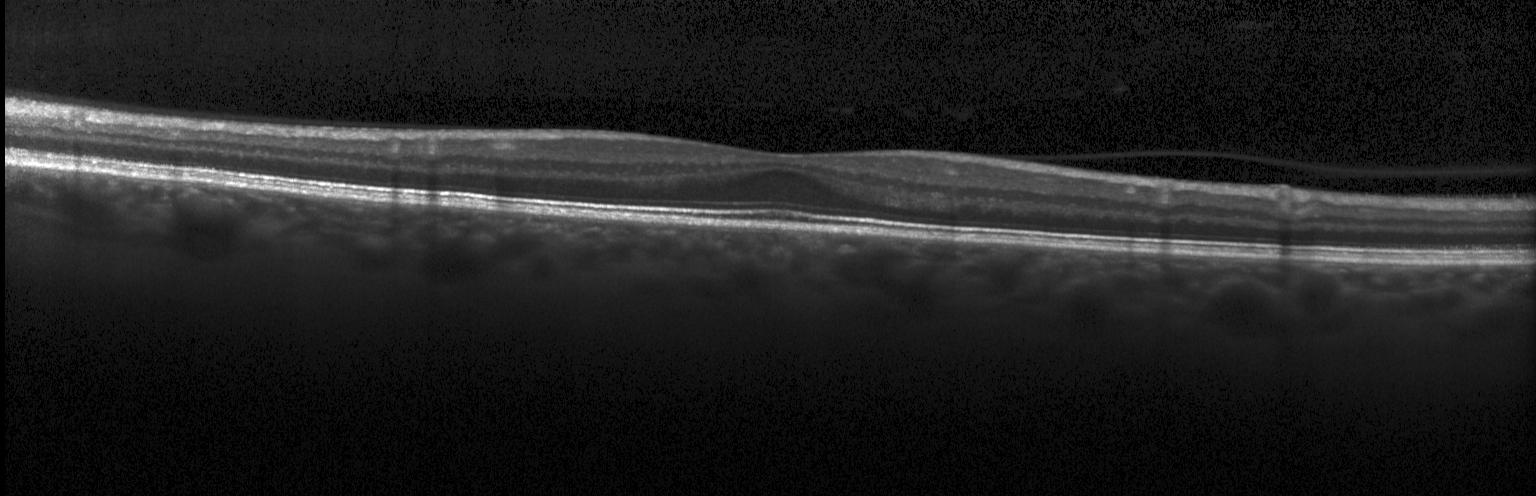

This B-scan demonstrates no evidence of CNV, DME, or drusen.